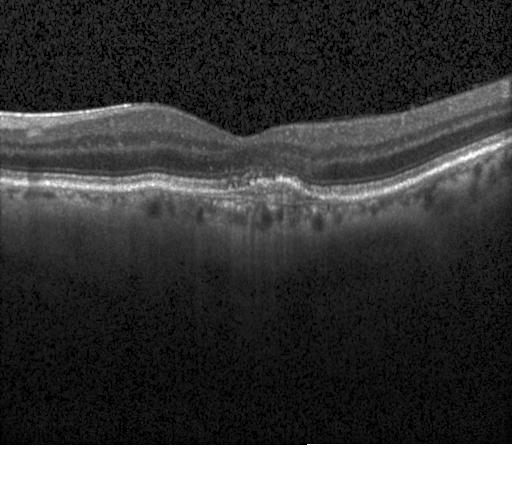
Spectral-domain OCT B-scan: a choroidal neovascular membrane.